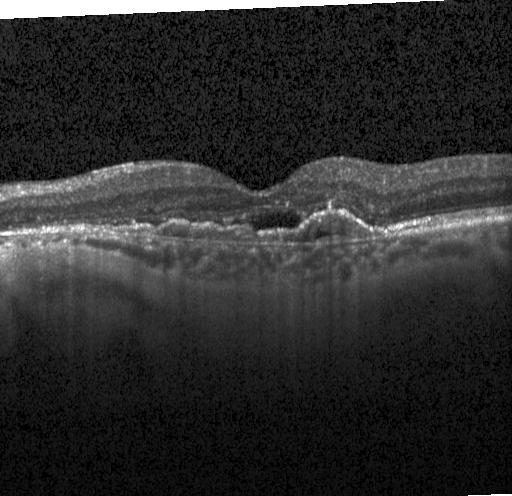

OCT line scan
Assessment: a choroidal neovascular membrane.